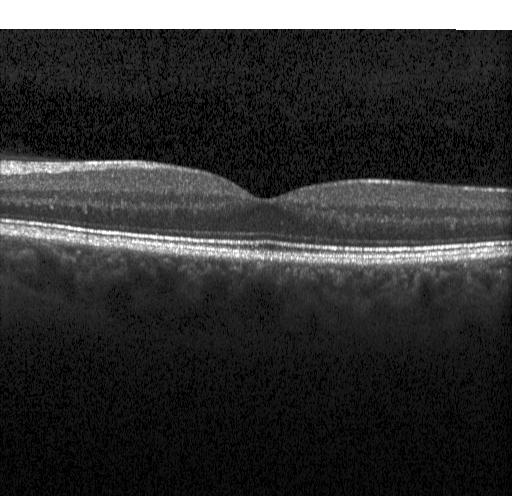

The scan shows no choroidal neovascularization, no diabetic macular edema, and no drusen.